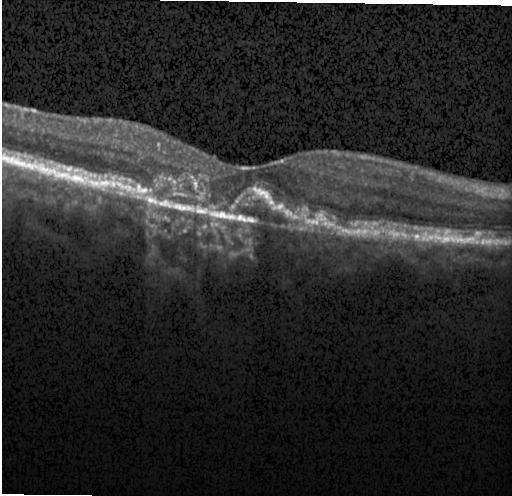 OCT B-scan.
Impression: choroidal neovascularization (CNV).